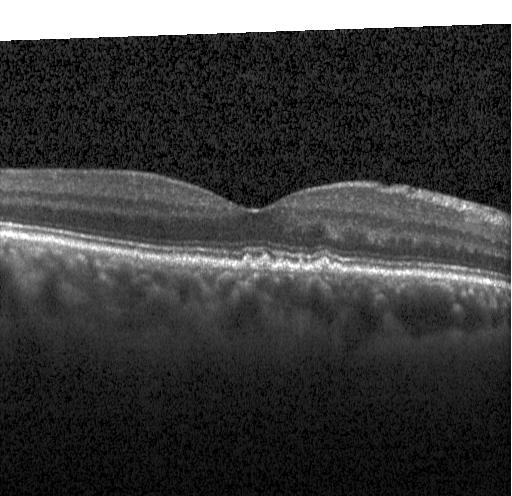 Macular OCT demonstrating multiple drusen.